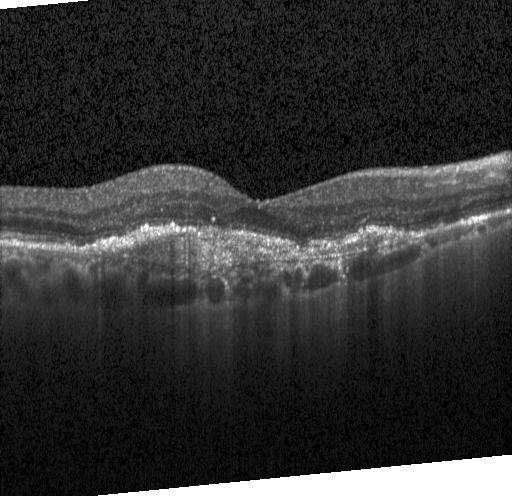

Optical coherence tomography scan, spectral-domain optical coherence tomography. Diagnosis: CNV.